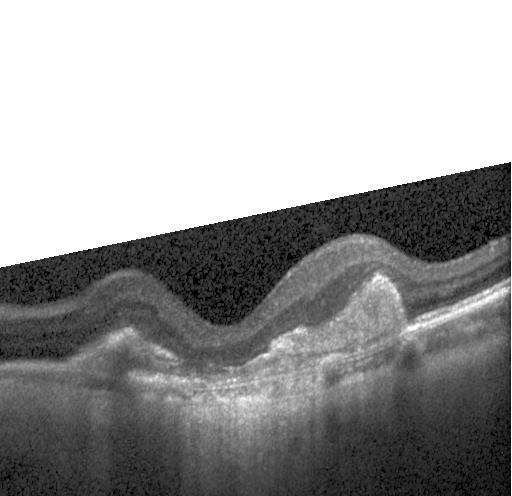

Retinal OCT B-scan · spectral-domain OCT · macular scan. Diagnosis: a choroidal neovascular membrane.